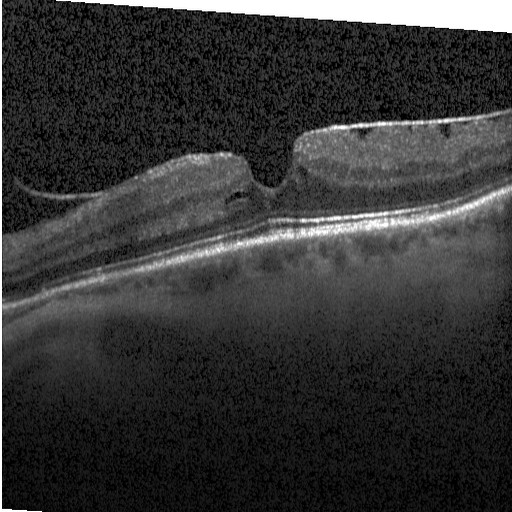

OCT line scan, Heidelberg Spectralis OCT system. The scan shows DME.